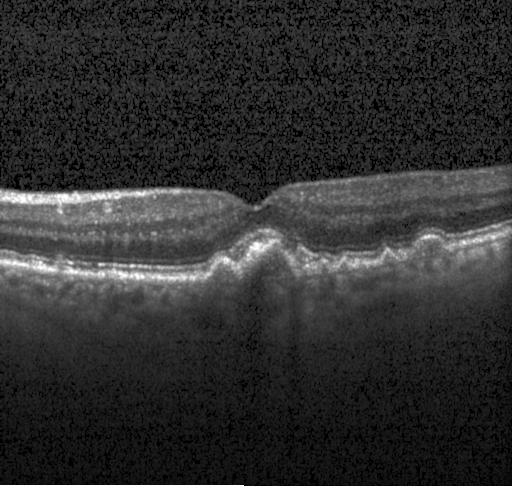 Impression: multiple drusen.